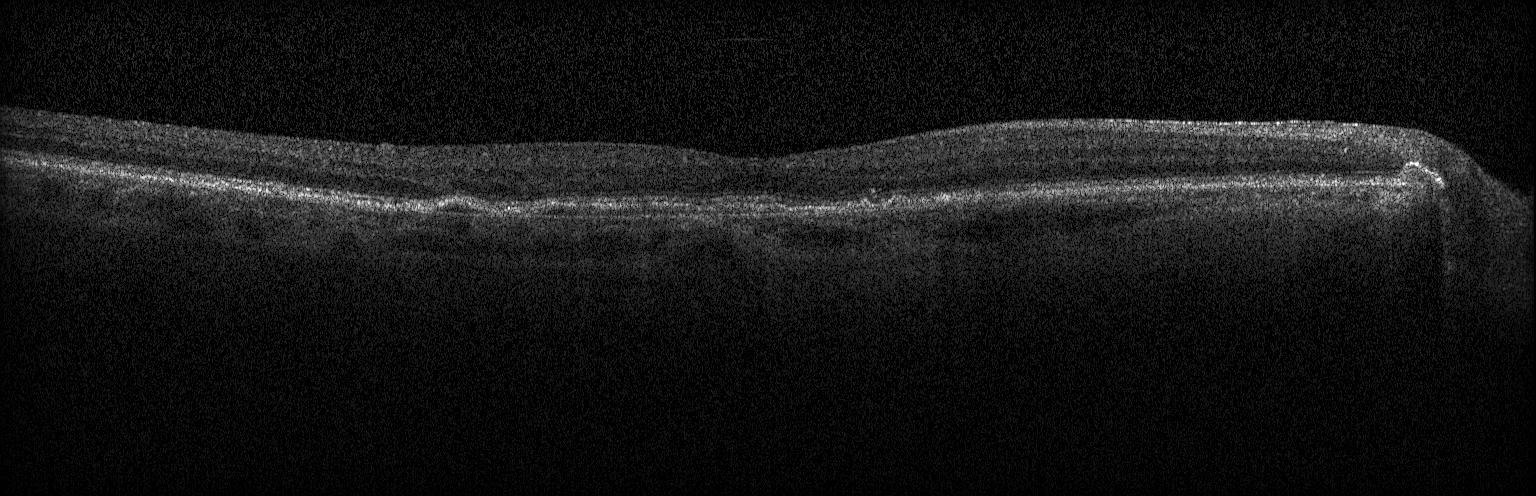
Retinal OCT cross-section showing a choroidal neovascular membrane.